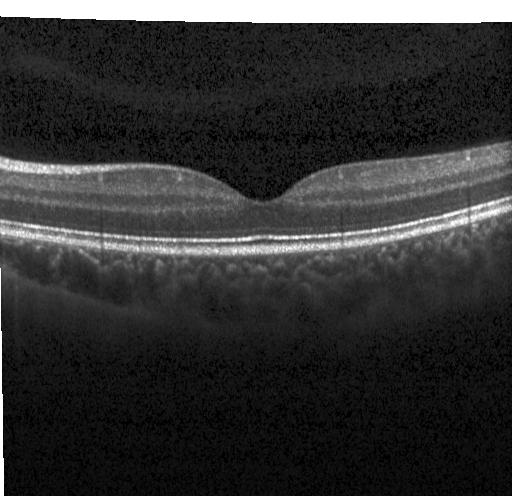

Macular OCT demonstrating no choroidal neovascularization, diabetic macular edema, or drusen.